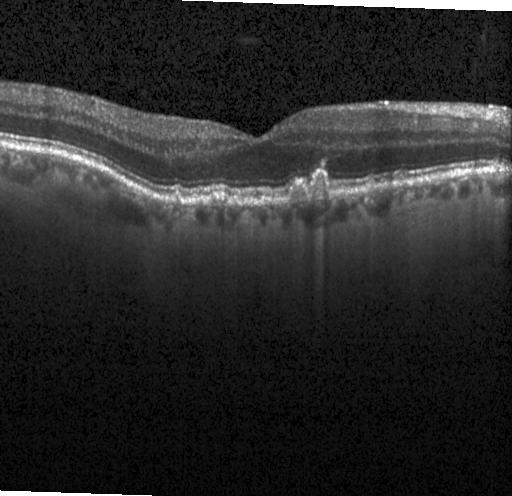

OCT line scan
Finding: sub-RPE drusenoid deposits.